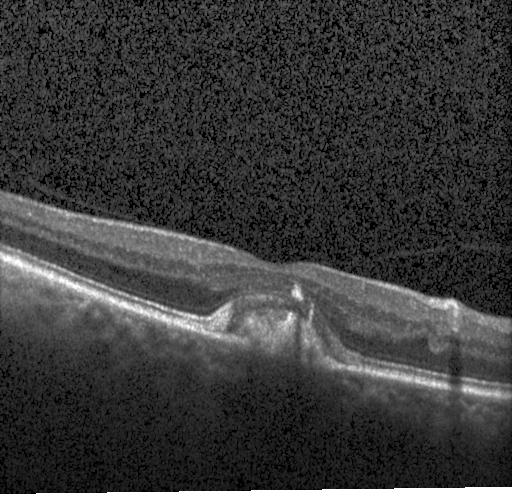 Spectral-domain OCT B-scan: a choroidal neovascular membrane.